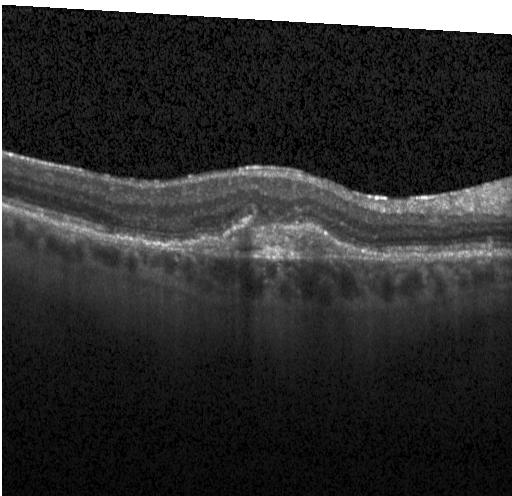
Centered on the fovea; instrument: Heidelberg Spectralis; spectral-domain optical coherence tomography; optical coherence tomography scan. The scan shows choroidal neovascularization.